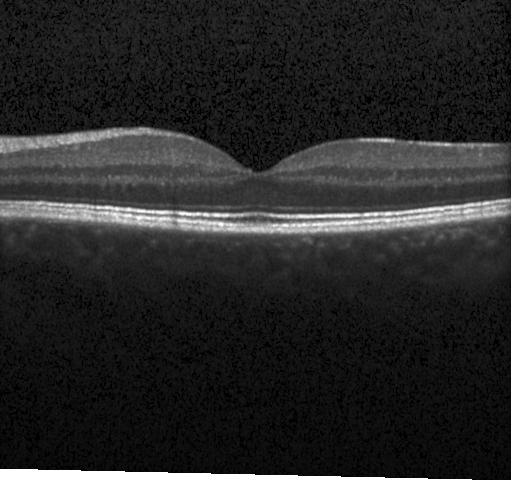

Acquired on a Heidelberg Spectralis, spectral-domain optical coherence tomography, OCT line scan, horizontal scan through the fovea. Finding: no choroidal neovascularization, no diabetic macular edema, and no drusen.